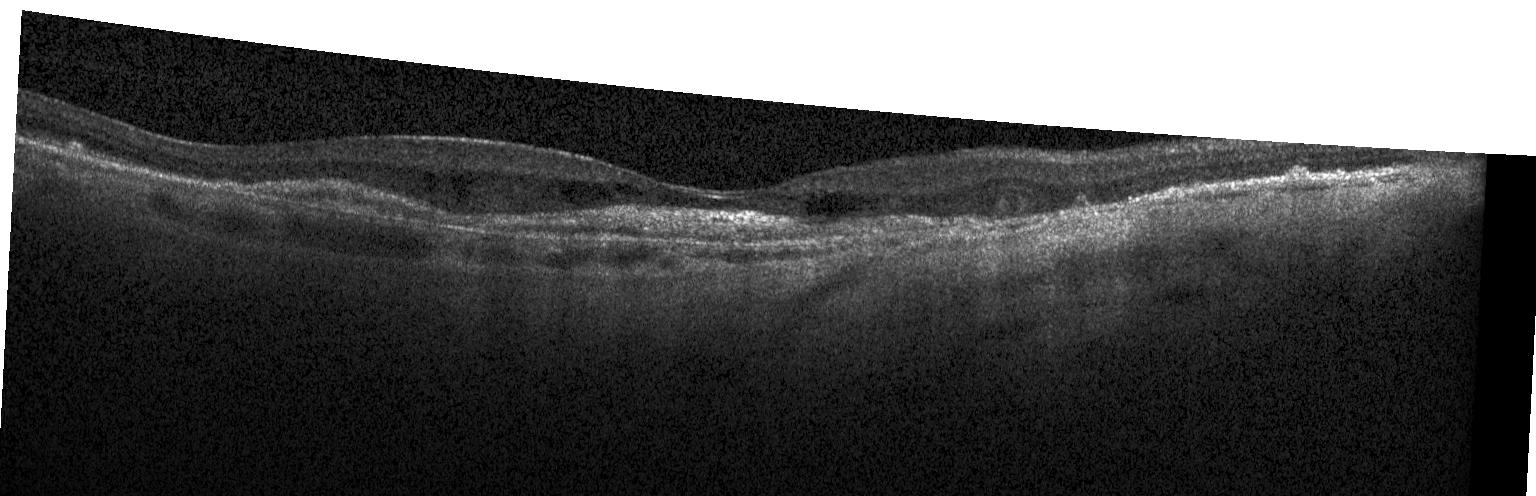 Heidelberg Spectralis OCT system, horizontal scan through the fovea, spectral-domain OCT, OCT B-scan
A choroidal neovascular membrane.